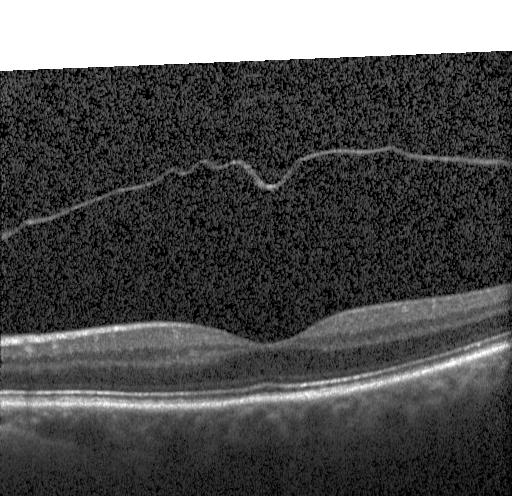 Finding: no evidence of choroidal neovascularization, diabetic macular edema, or drusen.